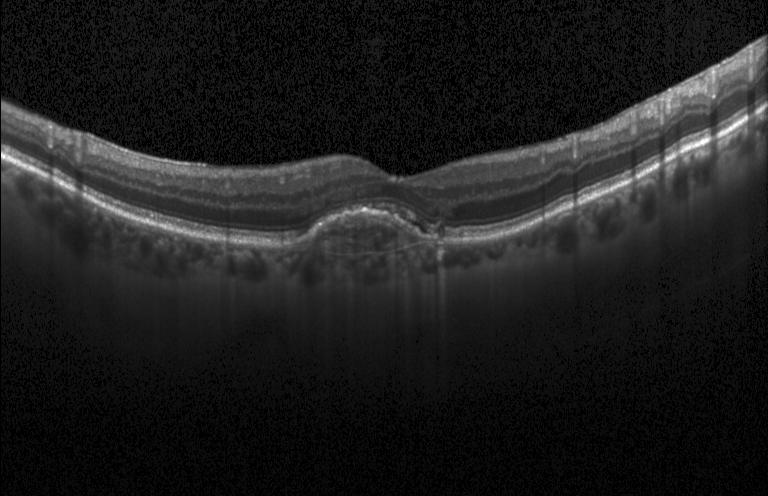 OCT line scan.
Macular OCT: choroidal neovascularization.